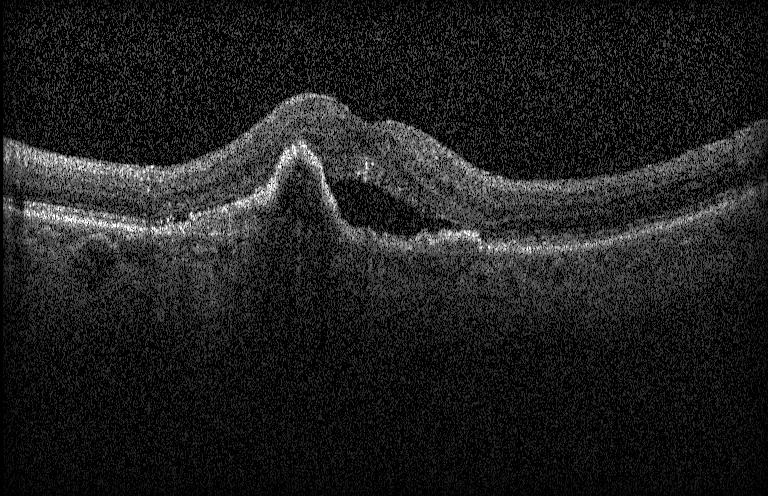
OCT B-scan — Diagnosis: CNV.